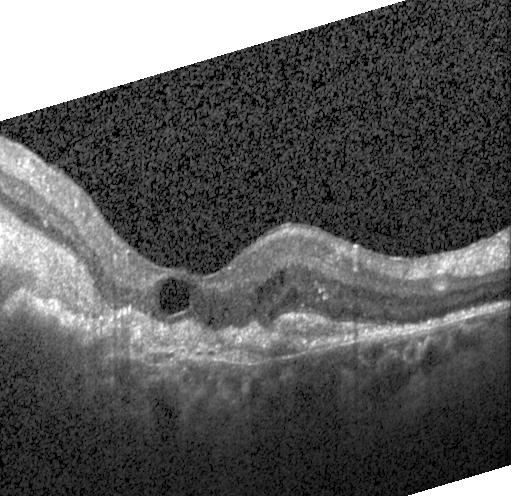
Spectral-domain optical coherence tomography · OCT B-scan · instrument: Heidelberg Spectralis · fovea-centered — Impression: CNV.